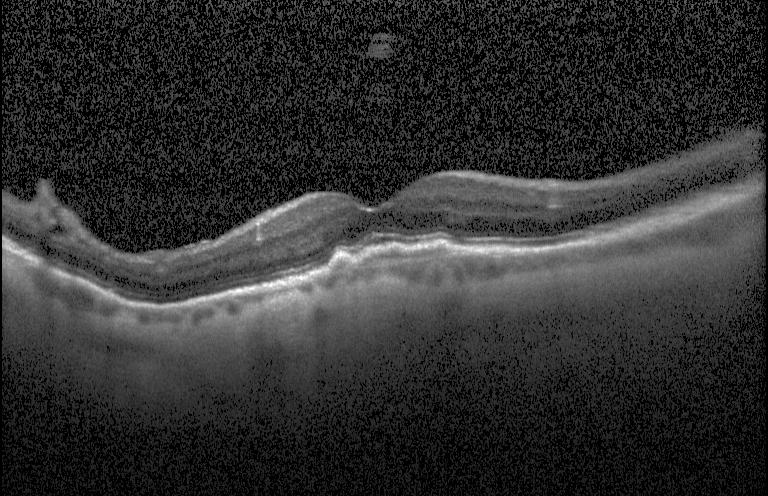
Fovea-centered · optical coherence tomography scan · spectral-domain OCT
The scan shows CNV.